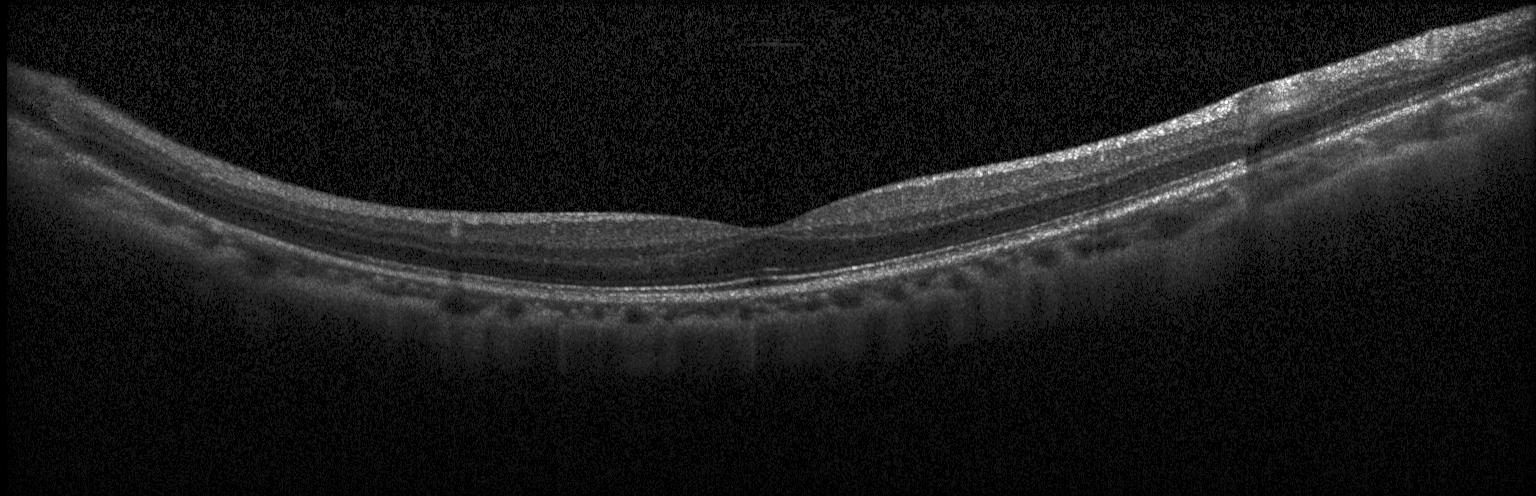
Finding: no CNV, DME, or drusen.